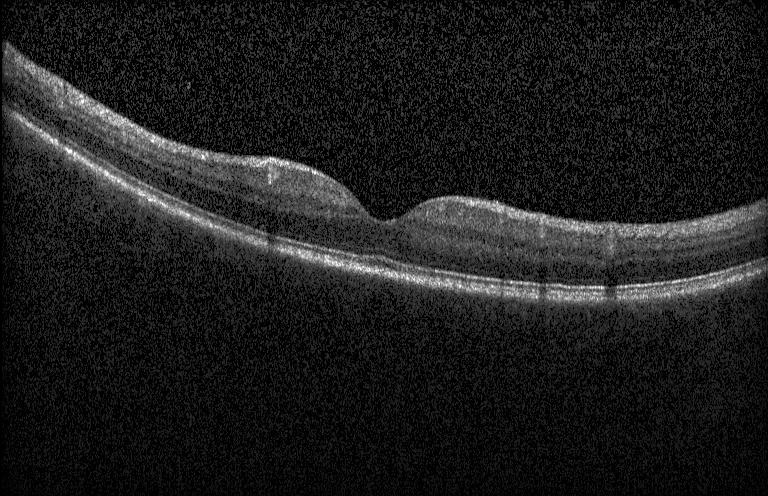
OCT scan showing no CNV, no DME, and no drusen.